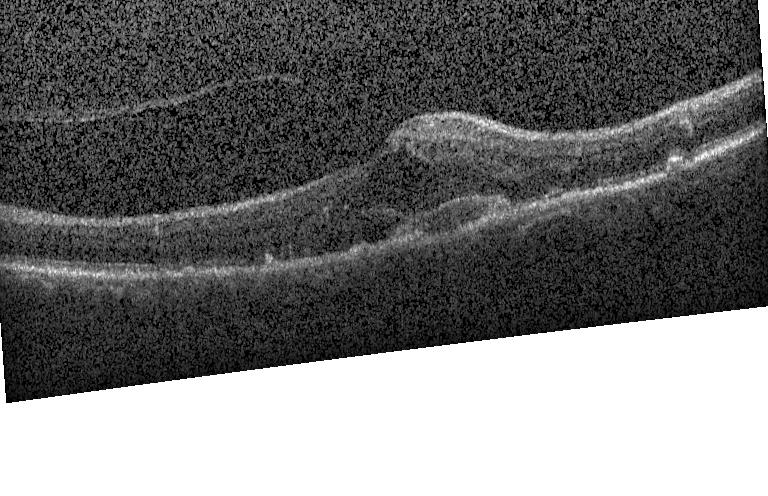
Retinal OCT B-scan
Diagnosis: choroidal neovascularization (CNV).